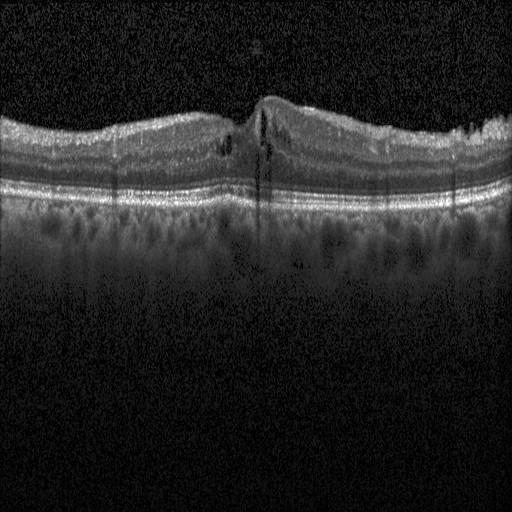 Retinal OCT cross-section. Assessment: diabetic macular edema.